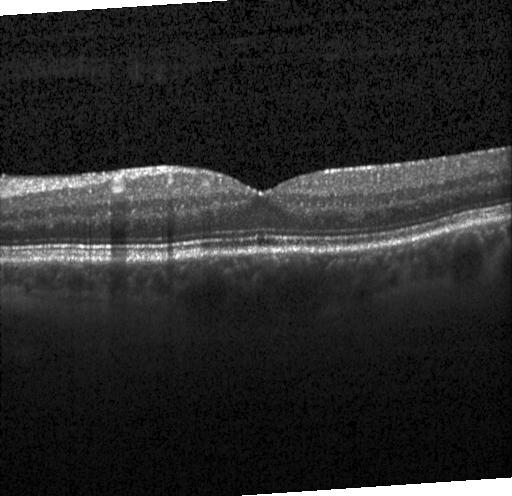

OCT line scan.
Finding: neither choroidal neovascularization, diabetic macular edema, nor drusen.